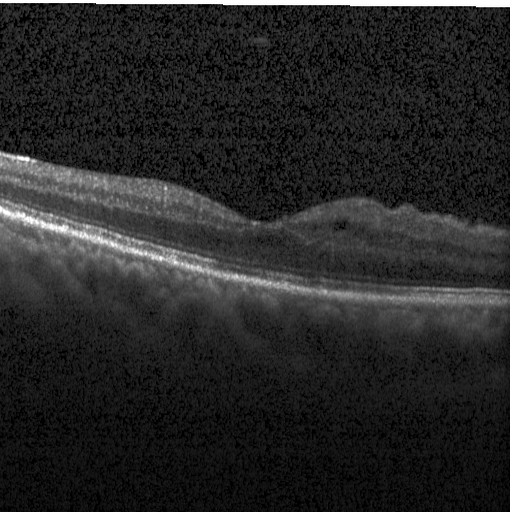
Finding: diabetic macular edema.